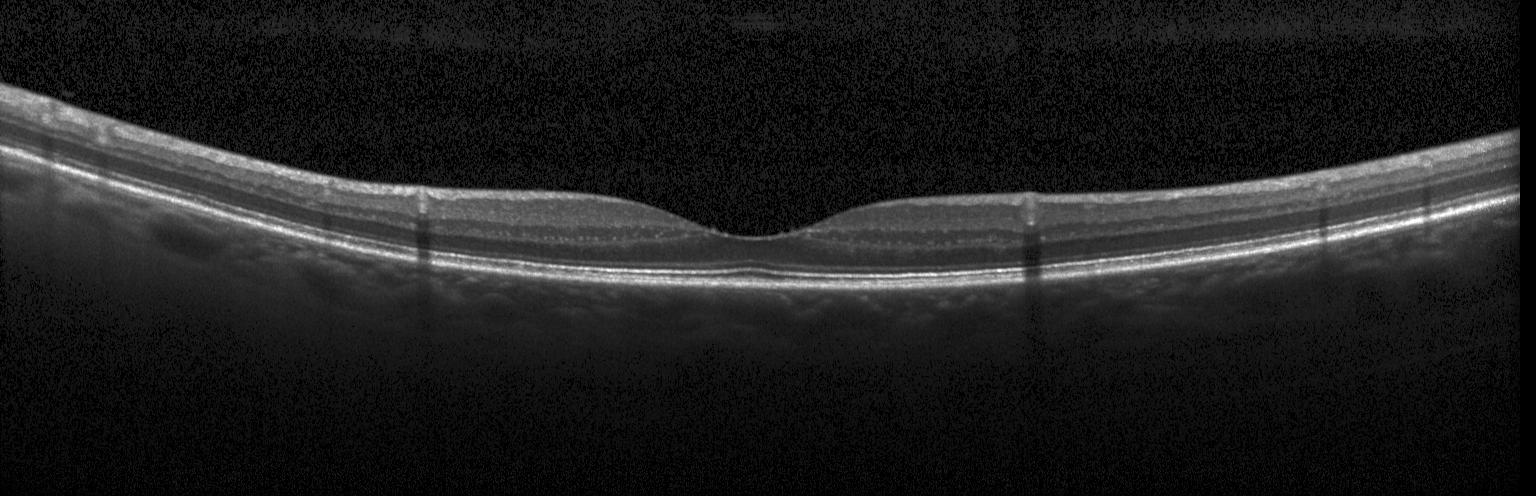

Retinal OCT cross-section
Dx: no choroidal neovascularization, no diabetic macular edema, and no drusen.